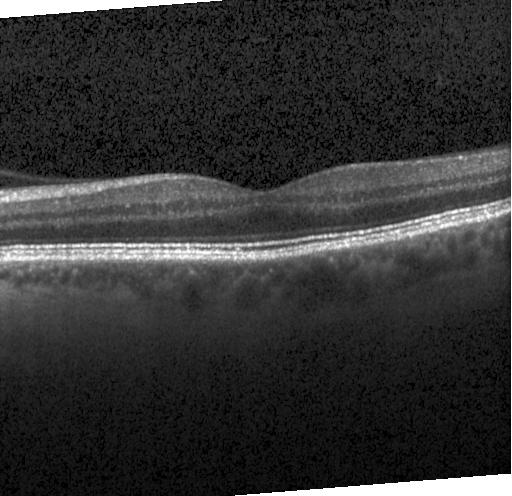

Macular OCT: no choroidal neovascularization, no diabetic macular edema, and no drusen.